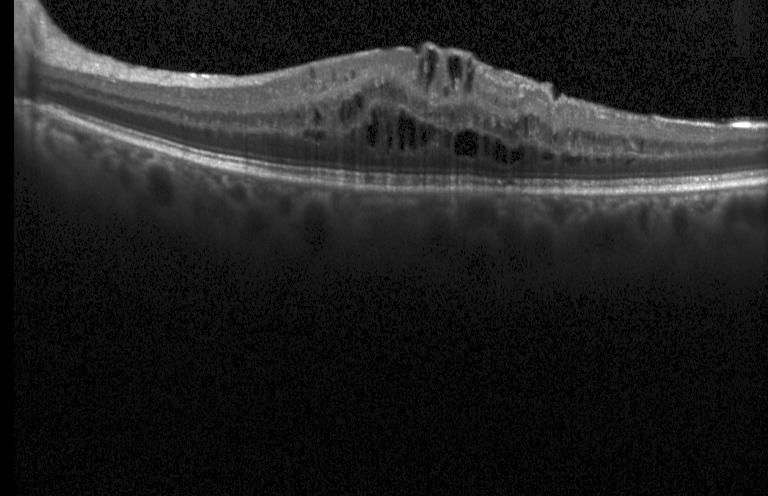 Finding: diabetic macular edema.